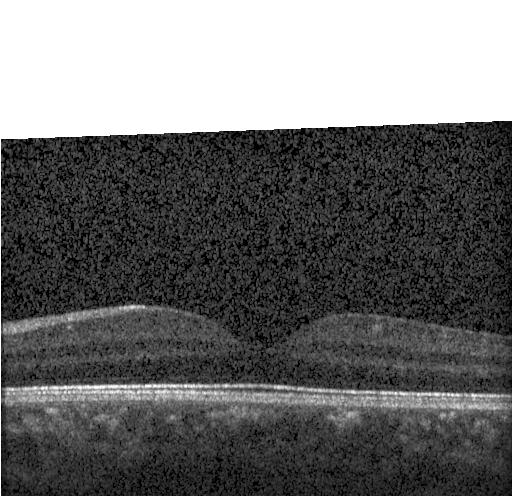

OCT B-scan showing no choroidal neovascularization, diabetic macular edema, or drusen.